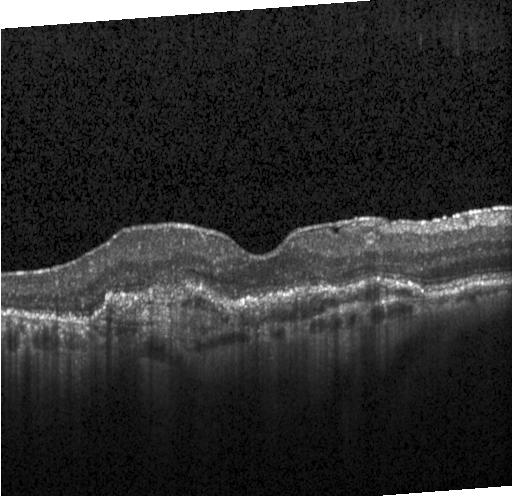

Finding: a choroidal neovascular membrane.